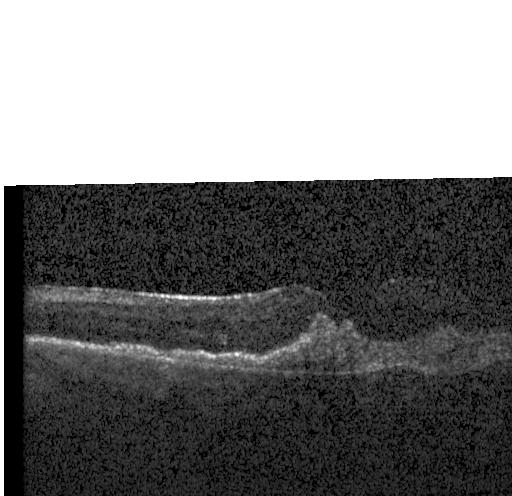

OCT scan showing a choroidal neovascular membrane.